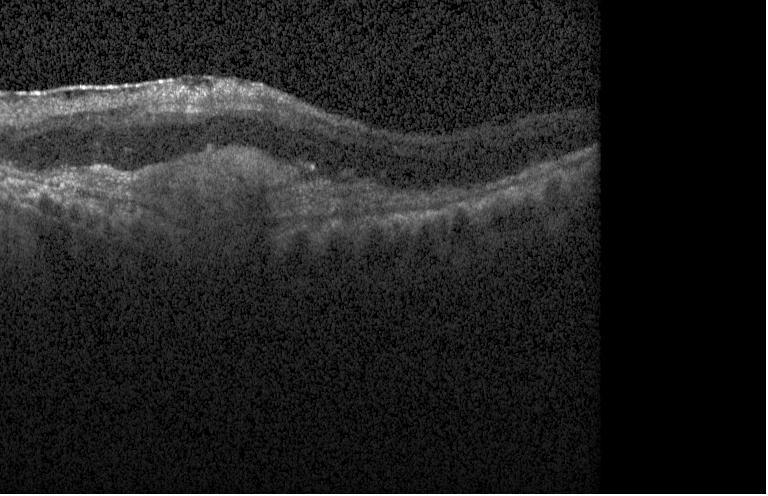

Optical coherence tomography scan, Heidelberg Spectralis, through the macula.
Macular OCT: choroidal neovascularization.